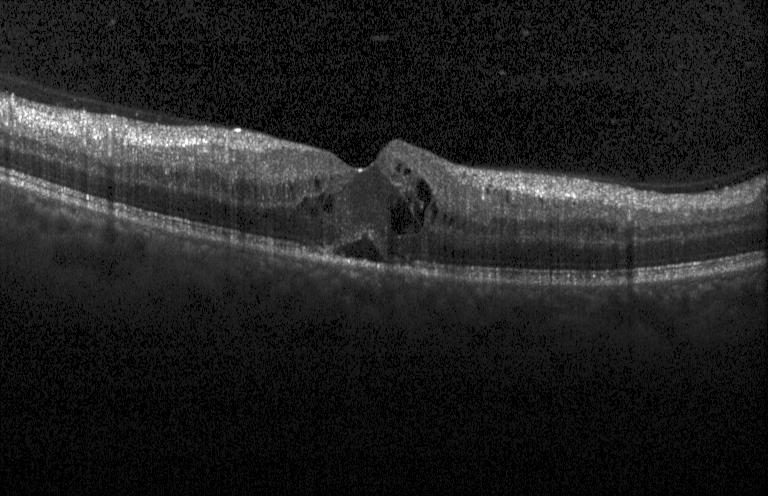 Finding: DME.